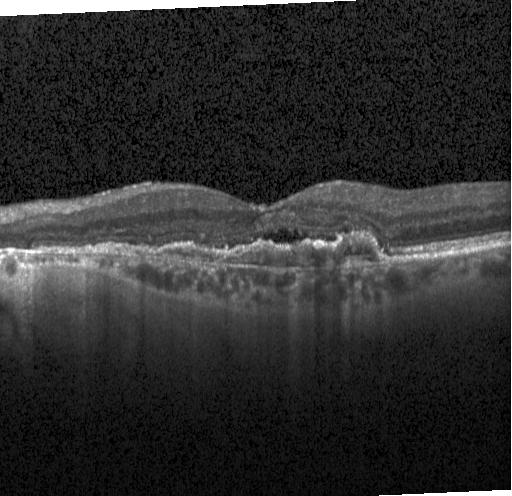
Heidelberg Spectralis OCT system. Centered on the fovea. SD-OCT. Optical coherence tomography B-scan.
CNV.